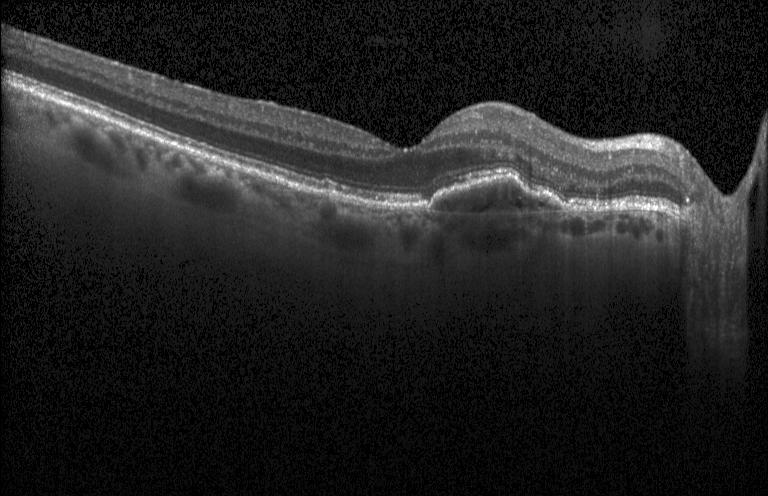

OCT B-scan
Macular OCT: choroidal neovascularization (CNV).